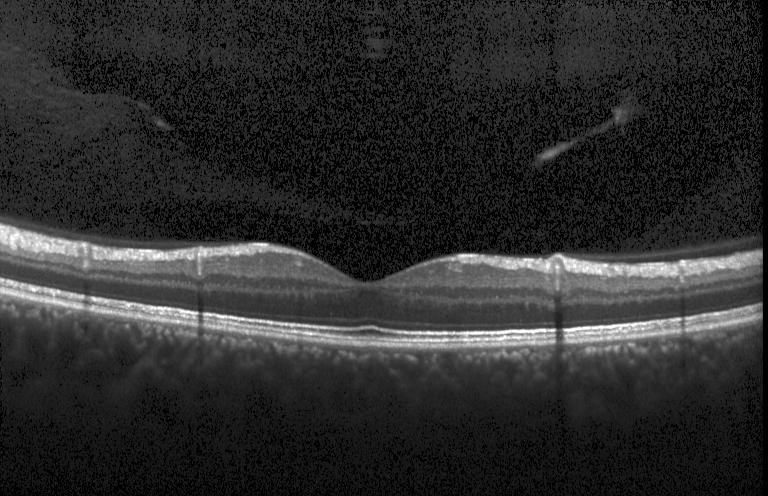 Fovea-centered. Spectral-domain optical coherence tomography. OCT B-scan. Heidelberg Spectralis OCT system. Diagnosis: no choroidal neovascularization, diabetic macular edema, or drusen.